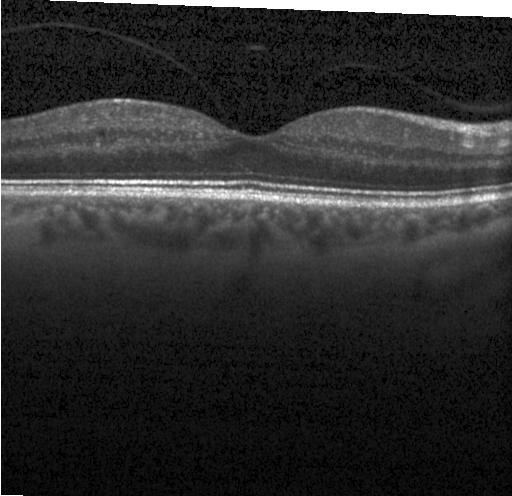
SD-OCT · fovea-centered · optical coherence tomography scan · instrument: Heidelberg Spectralis. Impression: DME.